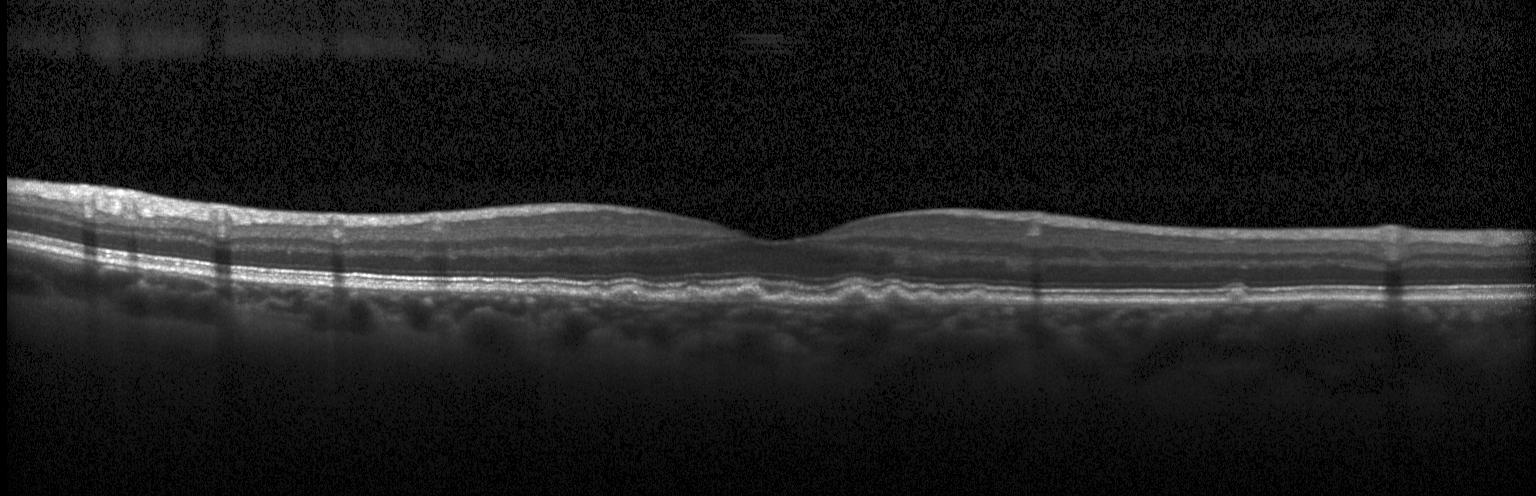

SD-OCT. Optical coherence tomography B-scan
The scan shows multiple drusen.